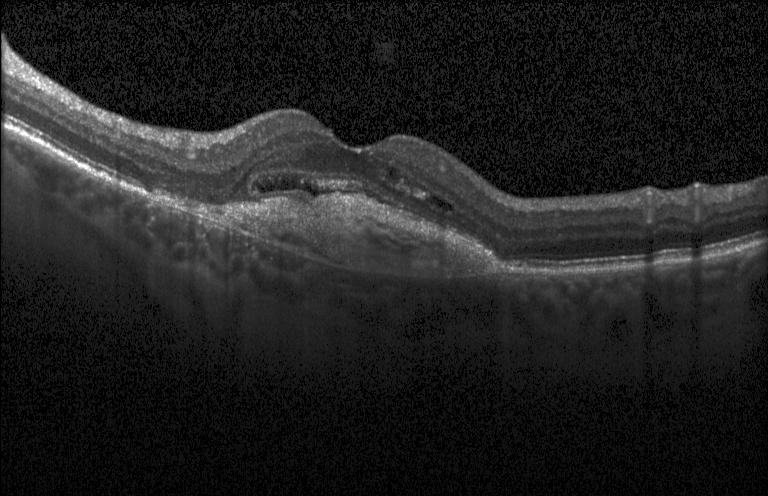
Optical coherence tomography B-scan. A choroidal neovascular membrane.